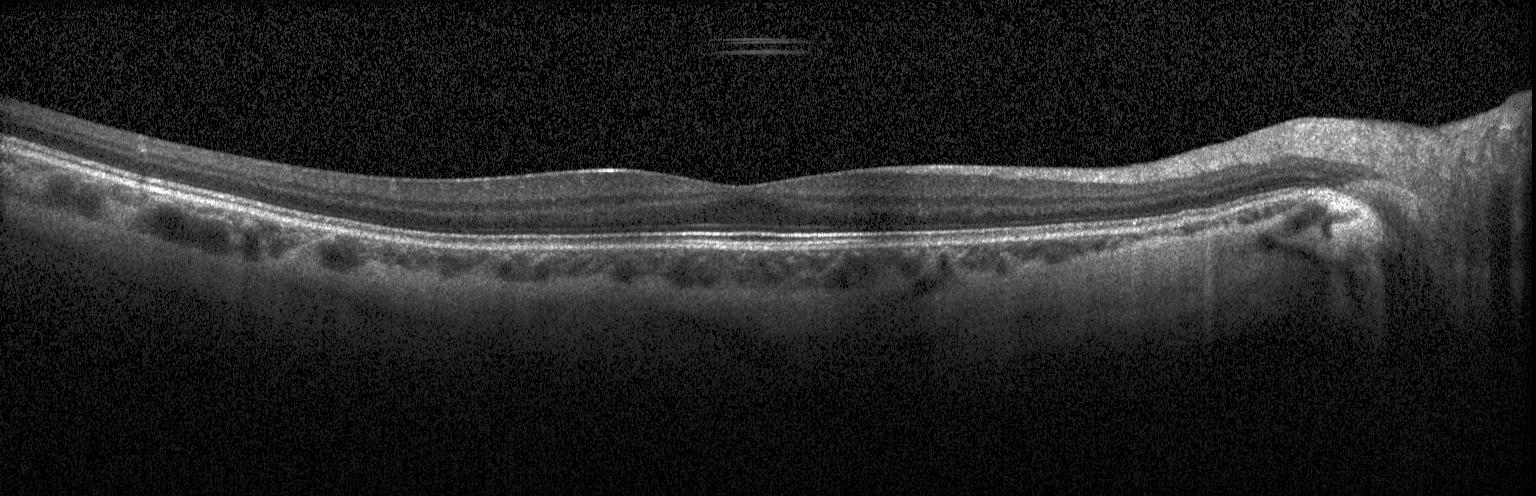

OCT line scan · instrument: Heidelberg Spectralis · spectral-domain optical coherence tomography · macular scan. OCT finding: neither CNV, DME, nor drusen.